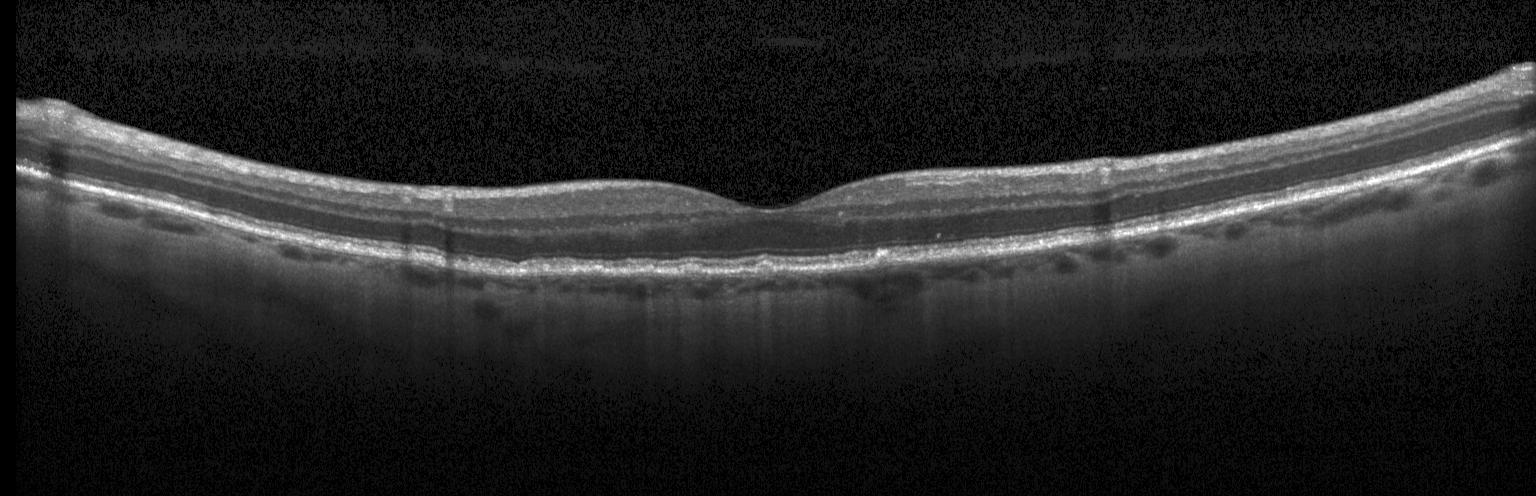

Retinal OCT B-scan; instrument: Heidelberg Spectralis.
Impression: drusen.